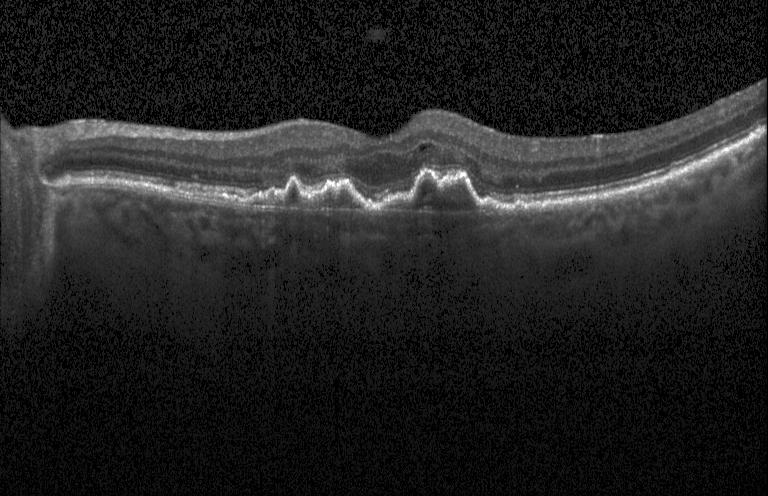 Spectral-domain optical coherence tomography. Retinal OCT B-scan. Acquired on a Heidelberg Spectralis
Impression: a choroidal neovascular membrane.